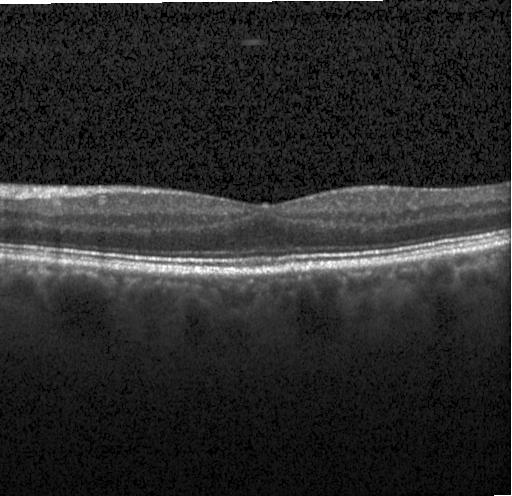
Heidelberg Spectralis OCT system; OCT B-scan — Neither choroidal neovascularization, diabetic macular edema, nor drusen.